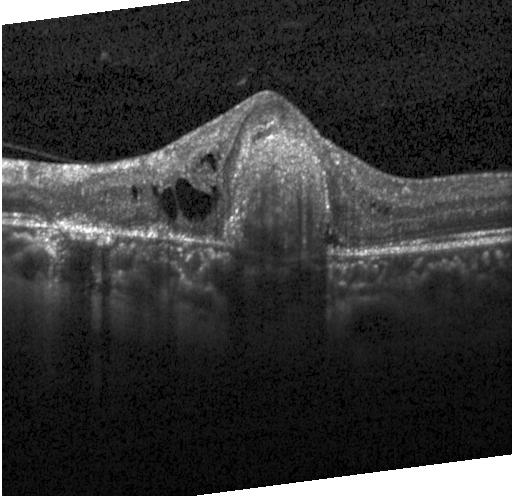 Dx: a choroidal neovascular membrane.